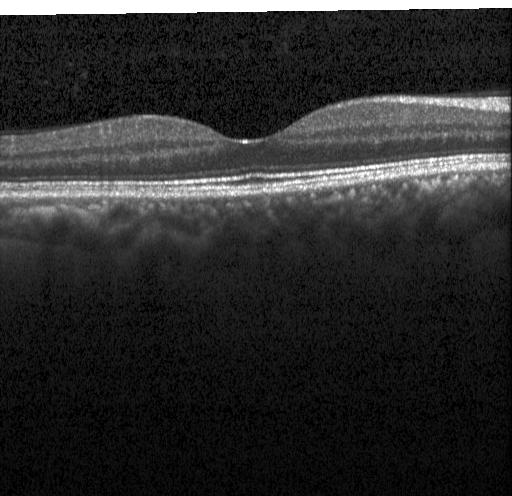 Retinal OCT cross-section showing neither choroidal neovascularization, diabetic macular edema, nor drusen.